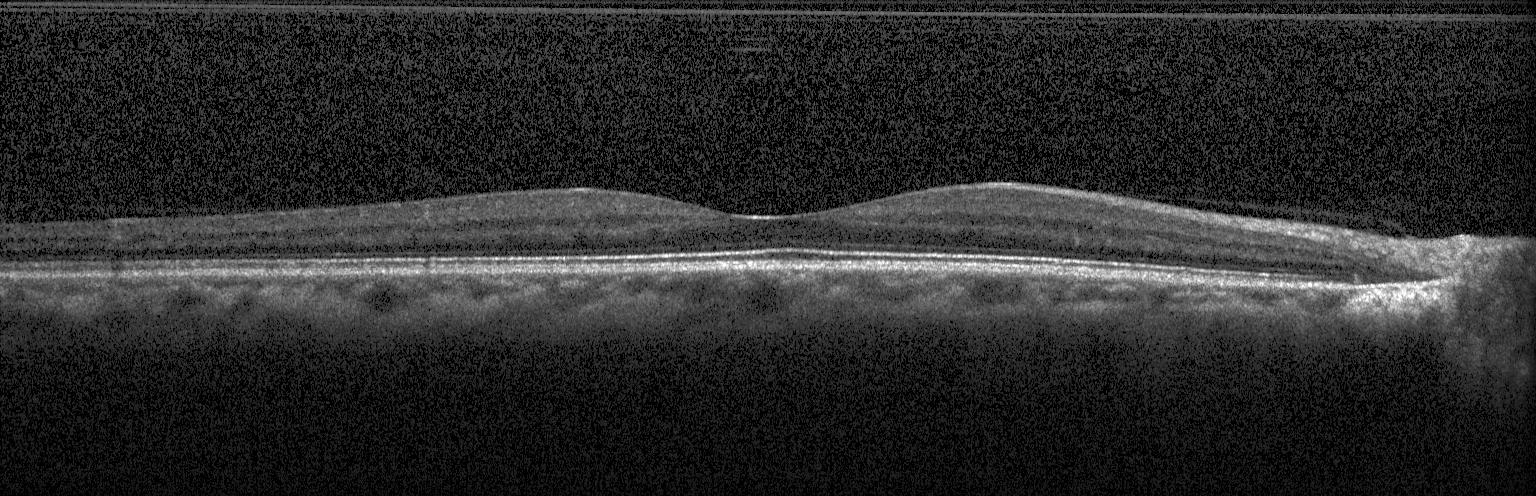 The scan shows neither choroidal neovascularization, diabetic macular edema, nor drusen.